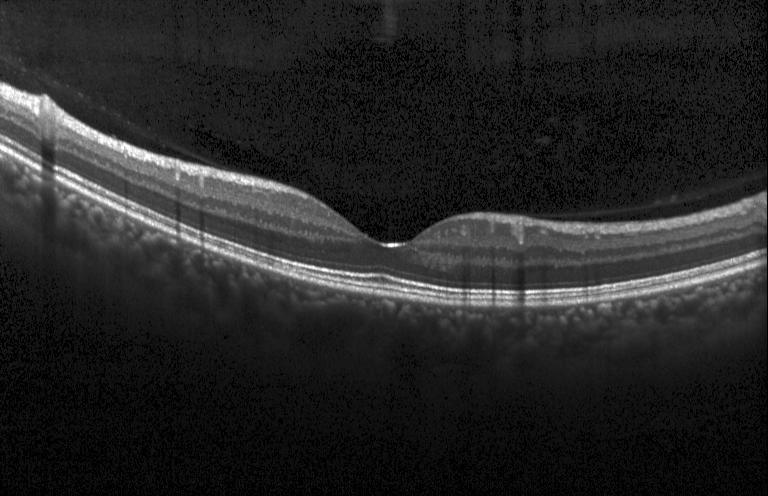
Macular OCT: no choroidal neovascularization, no diabetic macular edema, and no drusen.